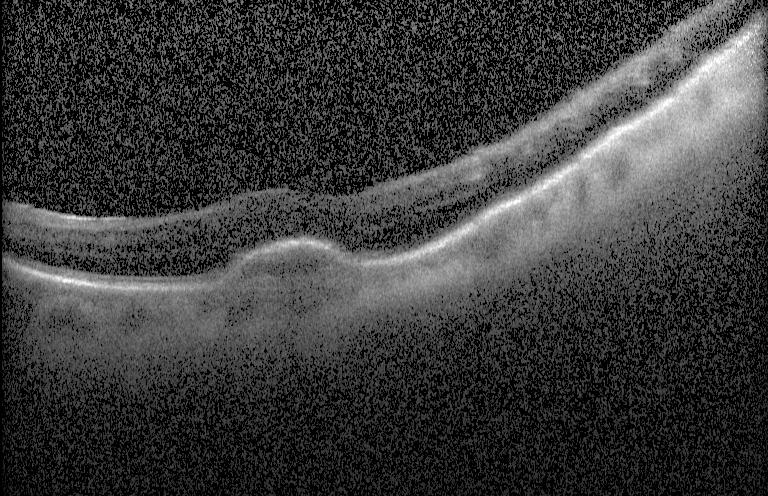

Optical coherence tomography scan. Macular scan. Heidelberg Spectralis OCT system. Macular OCT: a choroidal neovascular membrane.